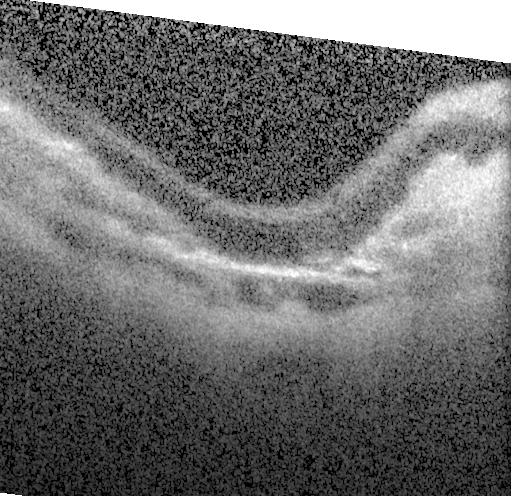 Macular OCT: choroidal neovascularization (CNV).